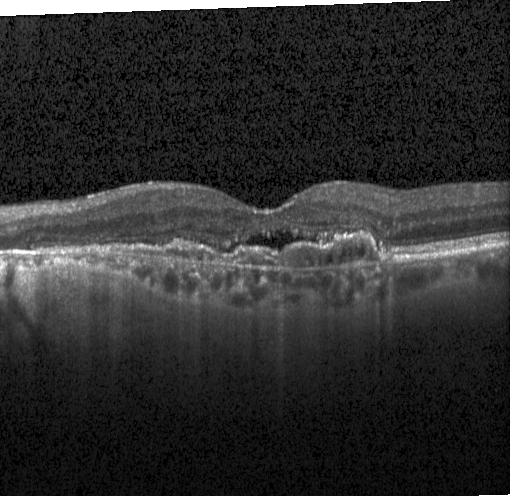
Retinal OCT cross-section. Choroidal neovascularization (CNV).